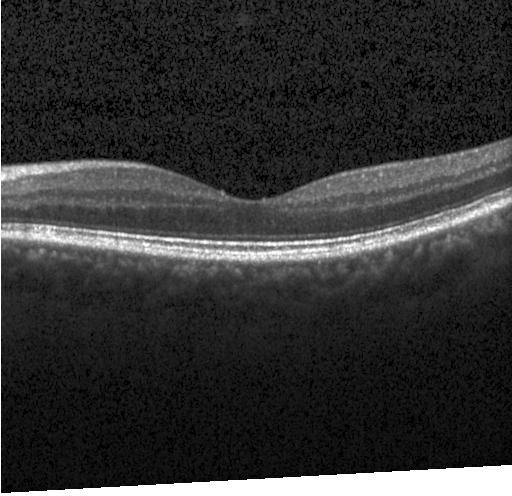

Retinal OCT B-scan
Assessment: no evidence of choroidal neovascularization, diabetic macular edema, or drusen.